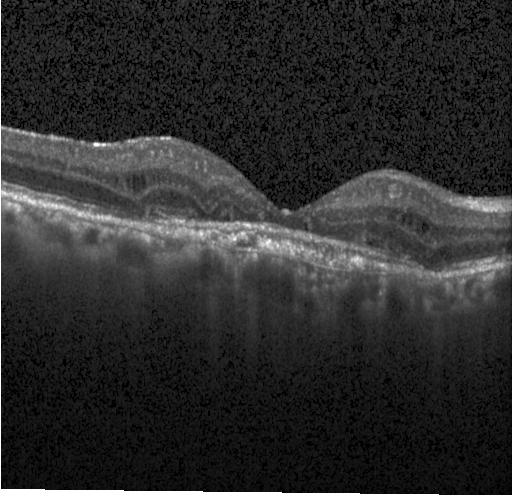

Diagnosis: a choroidal neovascular membrane.